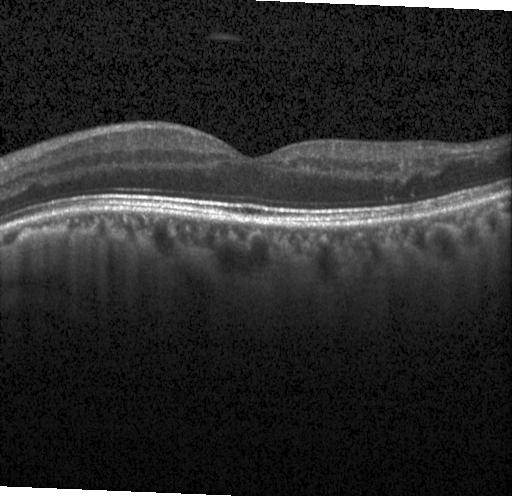

Optical coherence tomography scan.
Assessment: no evidence of CNV, DME, or drusen.